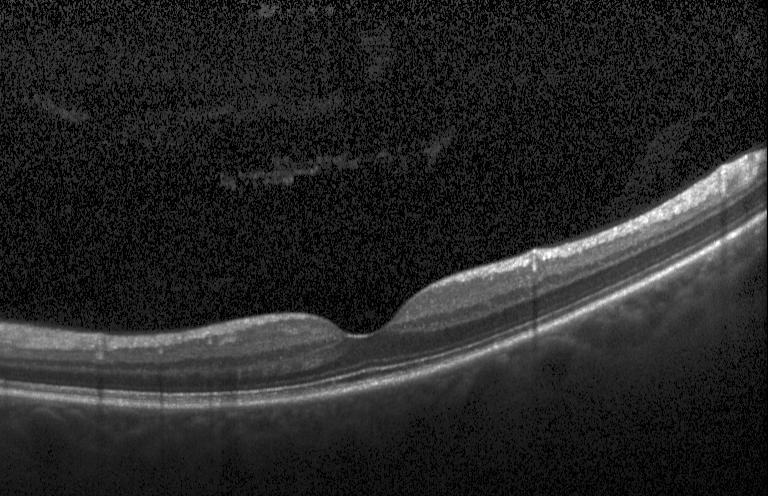

Macular scan · spectral-domain OCT · OCT line scan.
Neither choroidal neovascularization, diabetic macular edema, nor drusen.